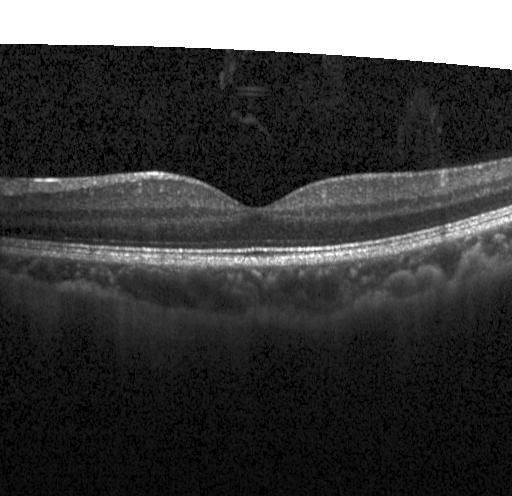 Optical coherence tomography B-scan. Impression: no evidence of choroidal neovascularization, diabetic macular edema, or drusen.